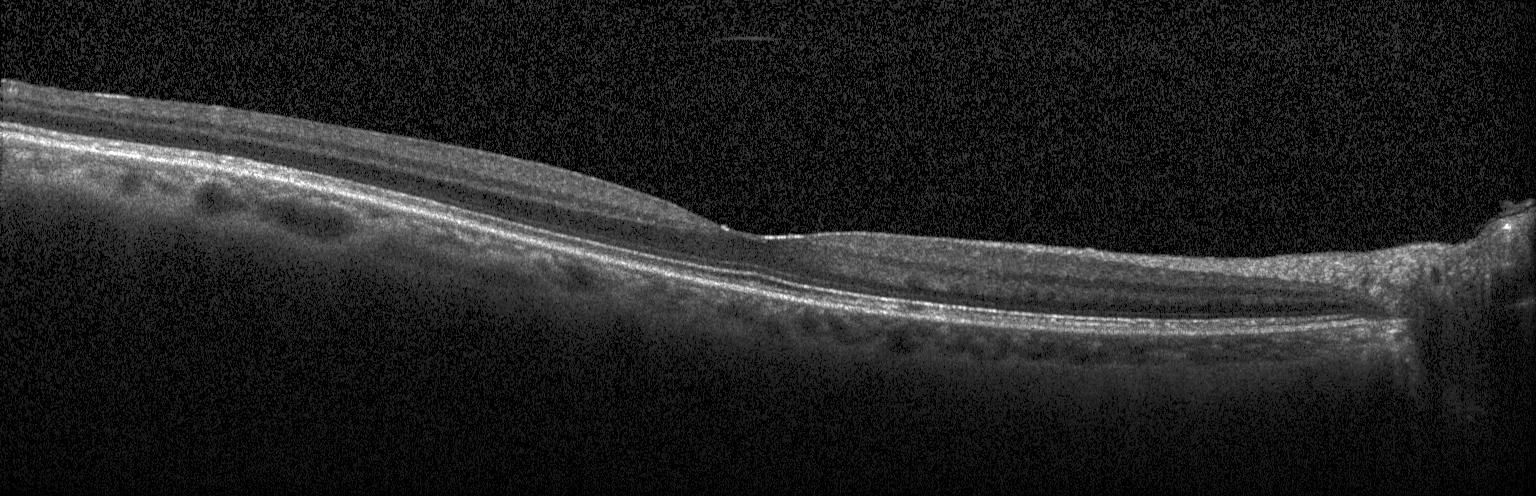 OCT scan showing no evidence of choroidal neovascularization, diabetic macular edema, or drusen.